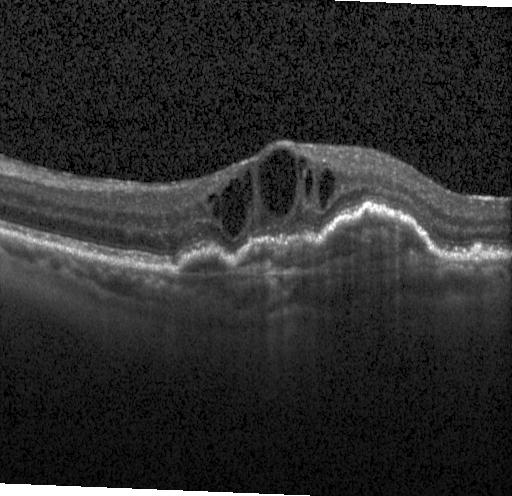

Retinal OCT cross-section — Dx: CNV.